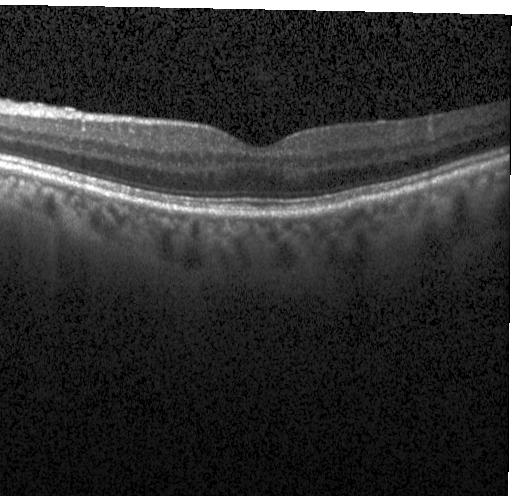 OCT line scan, fovea-centered.
Diagnosis: no choroidal neovascularization, diabetic macular edema, or drusen.